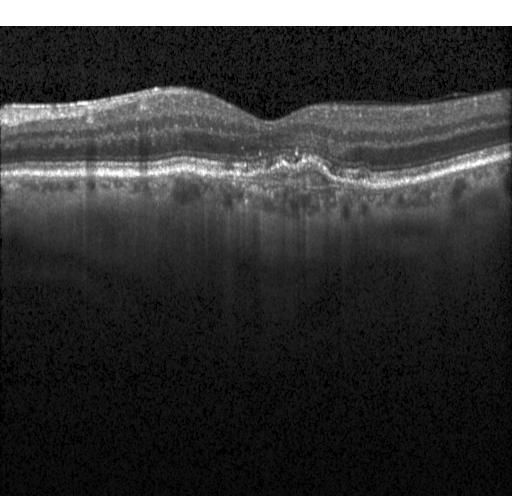
Spectral-domain OCT; fovea-centered; retinal OCT cross-section
Impression: CNV.